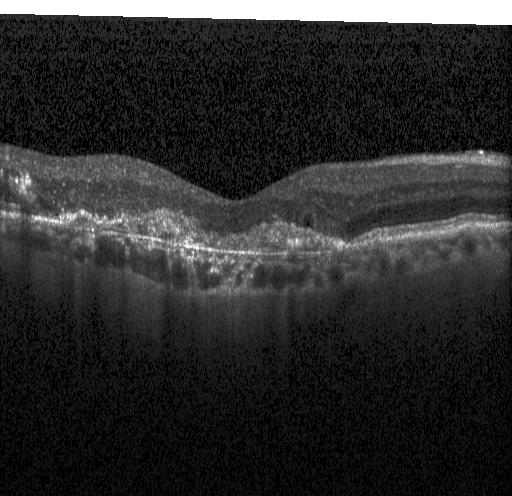
Macular scan, retinal OCT B-scan
Finding: CNV.